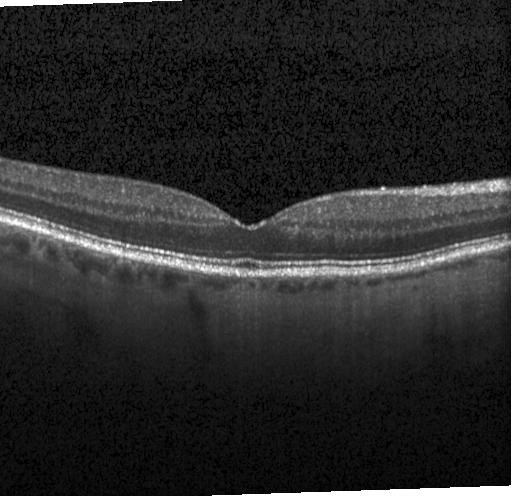 Retinal OCT cross-section showing no choroidal neovascularization, diabetic macular edema, or drusen.